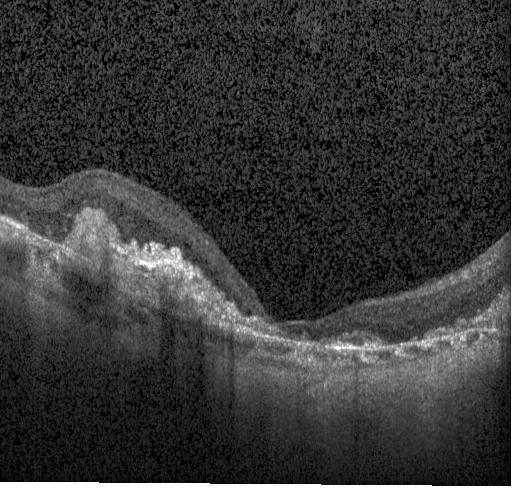
Dx: a choroidal neovascular membrane.